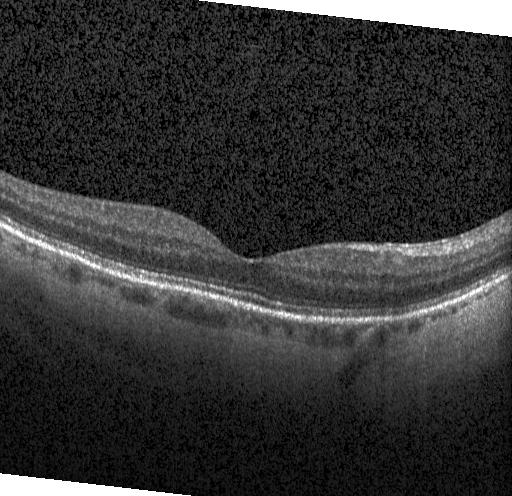
Optical coherence tomography B-scan
Impression: no evidence of CNV, DME, or drusen.